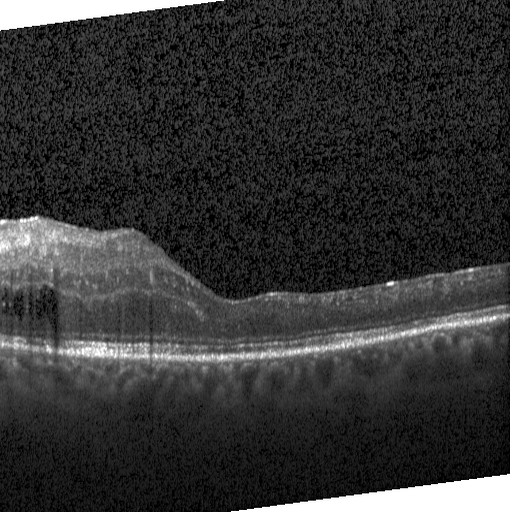 Heidelberg Spectralis OCT system, centered on the fovea, optical coherence tomography scan
Finding: DME.